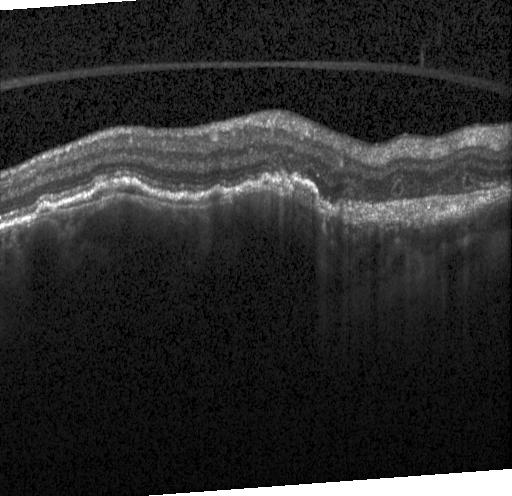 OCT B-scan
OCT finding: choroidal neovascularization (CNV).